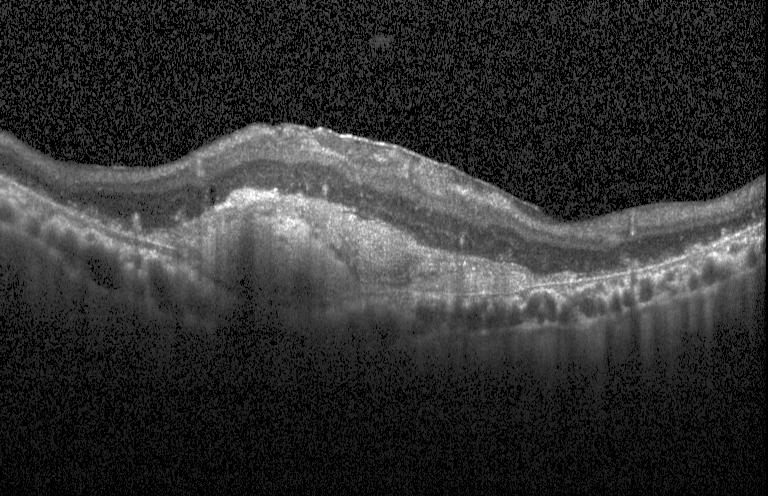

Impression: a choroidal neovascular membrane.